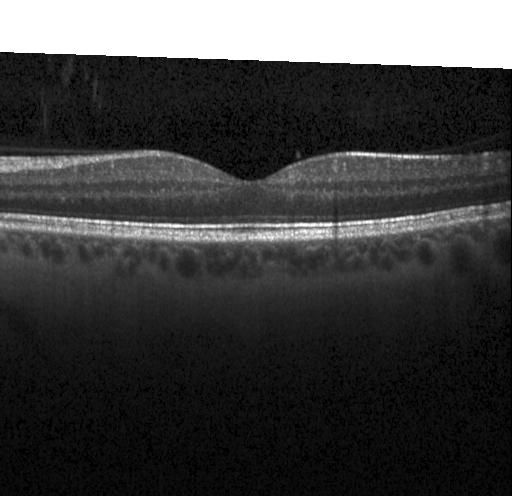

Macular scan · acquired on a Heidelberg Spectralis · OCT line scan. OCT finding: no choroidal neovascularization, no diabetic macular edema, and no drusen.